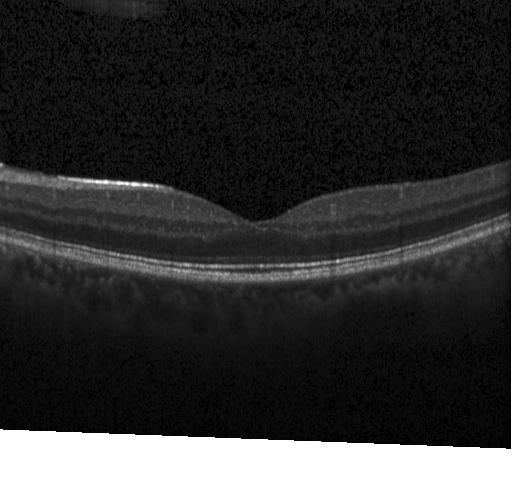

Centered on the fovea. Retinal OCT B-scan. Heidelberg Spectralis. Impression: no choroidal neovascularization, no diabetic macular edema, and no drusen.